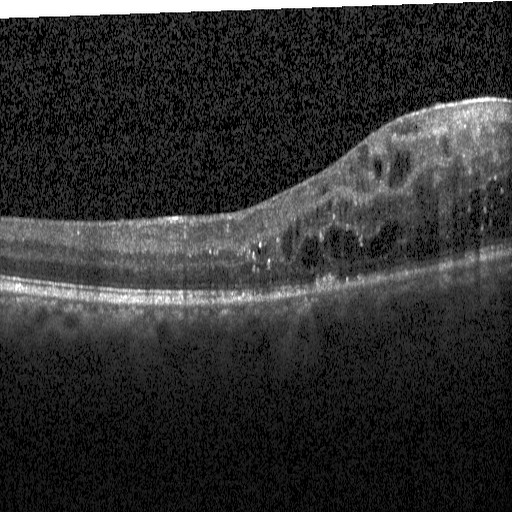
Spectral-domain OCT · optical coherence tomography B-scan · Heidelberg Spectralis · fovea-centered. This B-scan demonstrates diabetic macular edema.